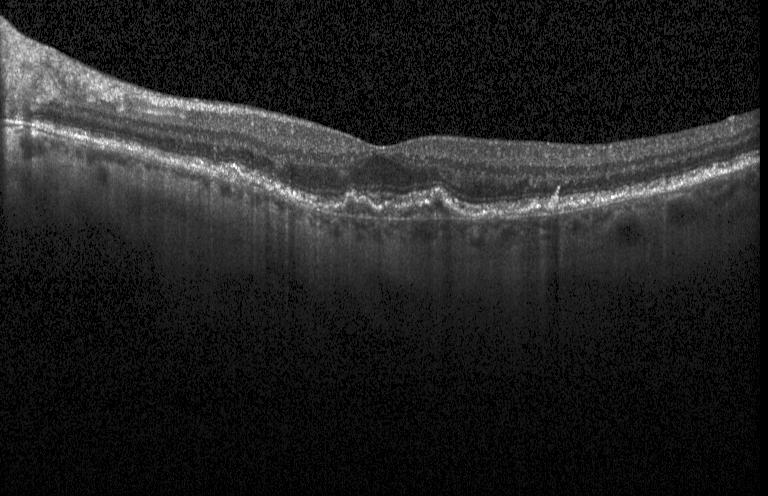 Dx: a choroidal neovascular membrane.